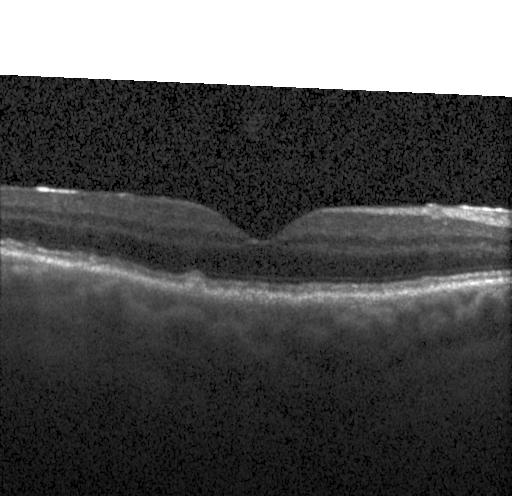

Horizontal scan through the fovea; acquired on a Heidelberg Spectralis; optical coherence tomography B-scan. OCT finding: sub-RPE drusenoid deposits.